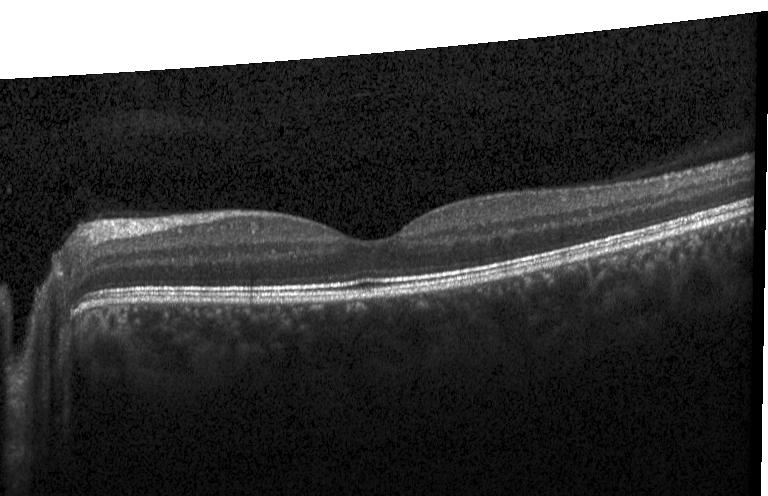 Horizontal scan through the fovea. OCT line scan. Instrument: Heidelberg Spectralis. SD-OCT
Dx: no evidence of choroidal neovascularization, diabetic macular edema, or drusen.